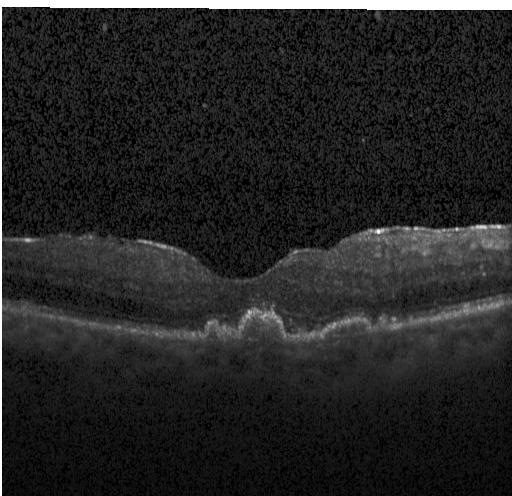
Finding: sub-RPE drusenoid deposits.